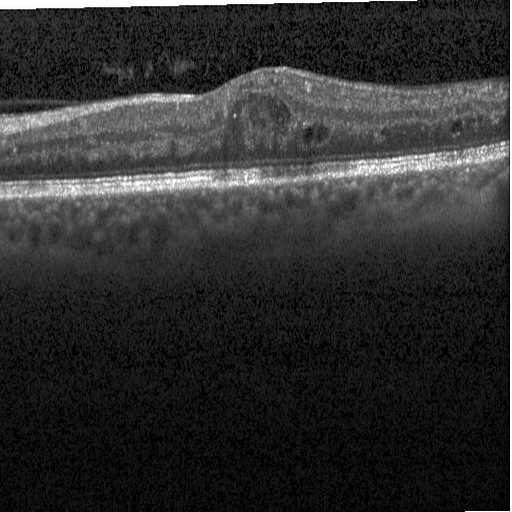

OCT line scan · Heidelberg Spectralis · SD-OCT · through the macula.
Diagnosis: diabetic macular edema (DME).